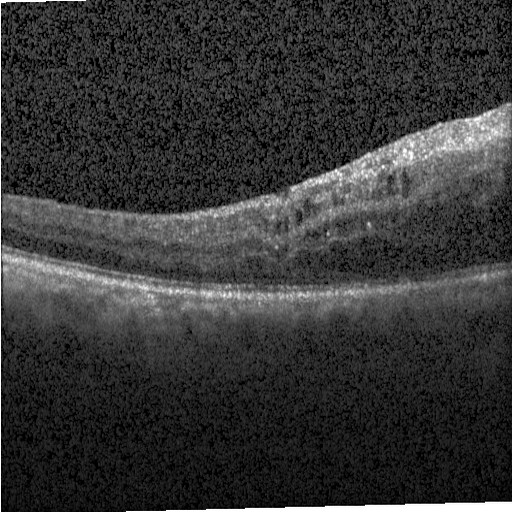

Optical coherence tomography scan, spectral-domain optical coherence tomography, through the macula.
Diagnosis: diabetic macular edema.